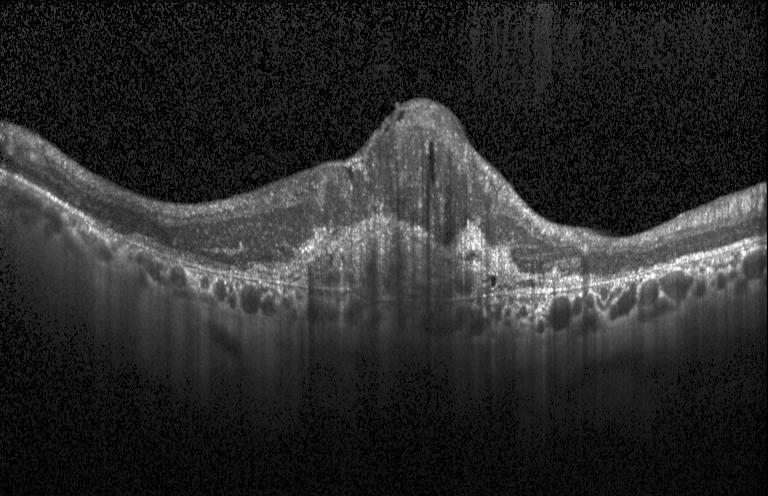 Optical coherence tomography B-scan. Diagnosis: choroidal neovascularization (CNV).